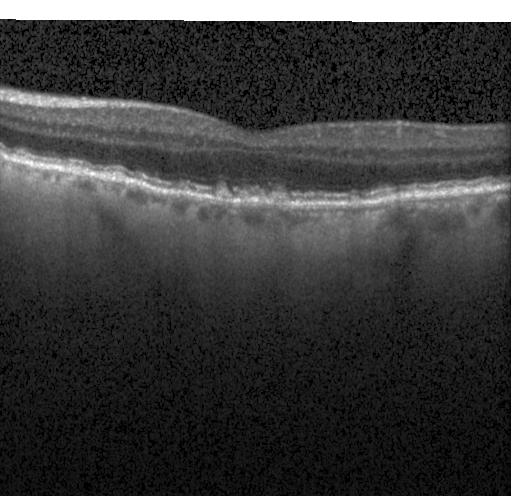 Retinal OCT B-scan. Heidelberg Spectralis OCT system
Diagnosis: sub-RPE drusenoid deposits.